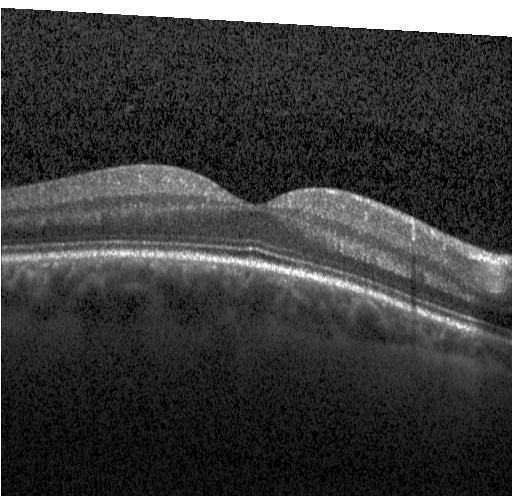

Retinal OCT cross-section showing no CNV, no DME, and no drusen.